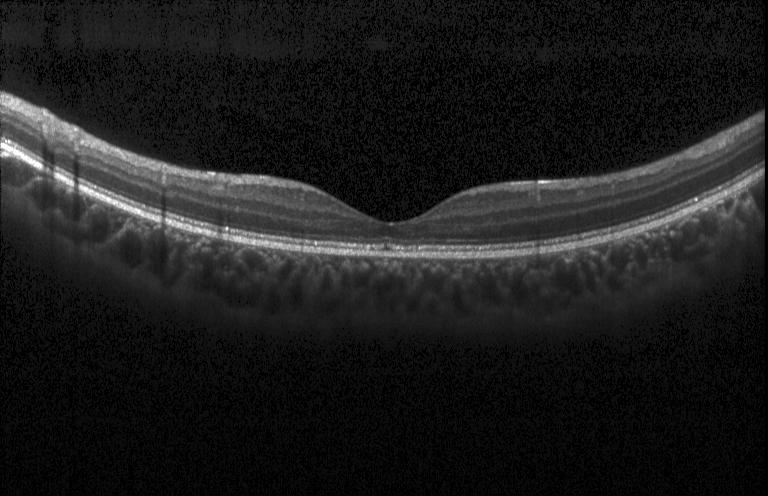

OCT B-scan showing no evidence of choroidal neovascularization, diabetic macular edema, or drusen.